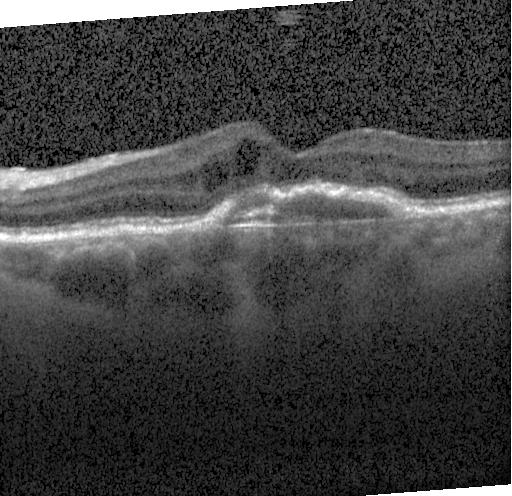
Assessment: a choroidal neovascular membrane.